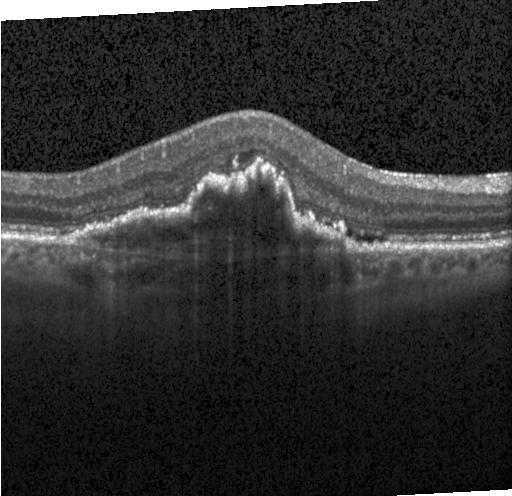 SD-OCT; centered on the fovea; optical coherence tomography scan
The scan shows CNV.